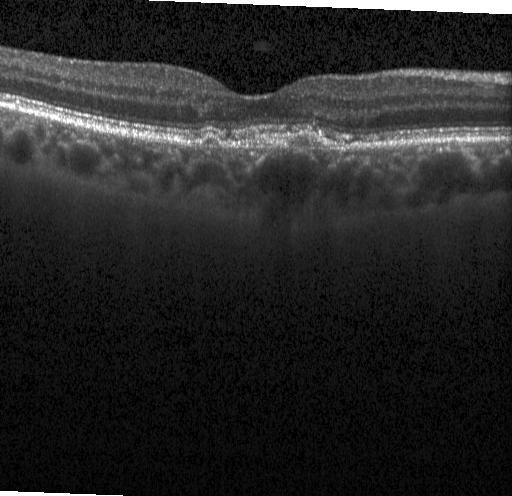

Retinal OCT B-scan · spectral-domain optical coherence tomography · acquired on a Heidelberg Spectralis. Dx: choroidal neovascularization.